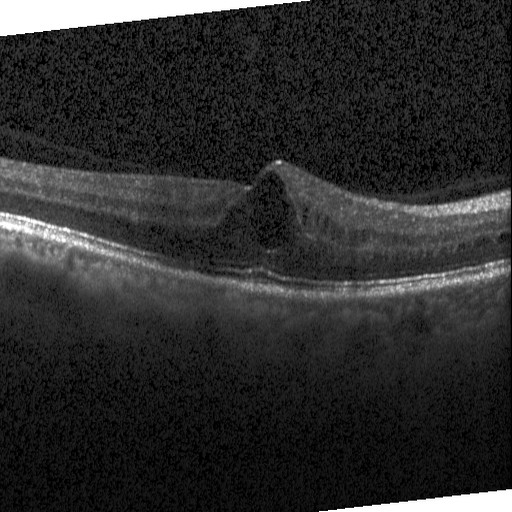 Instrument: Heidelberg Spectralis; SD-OCT; fovea-centered; optical coherence tomography scan.
Dx: diabetic macular edema (DME).